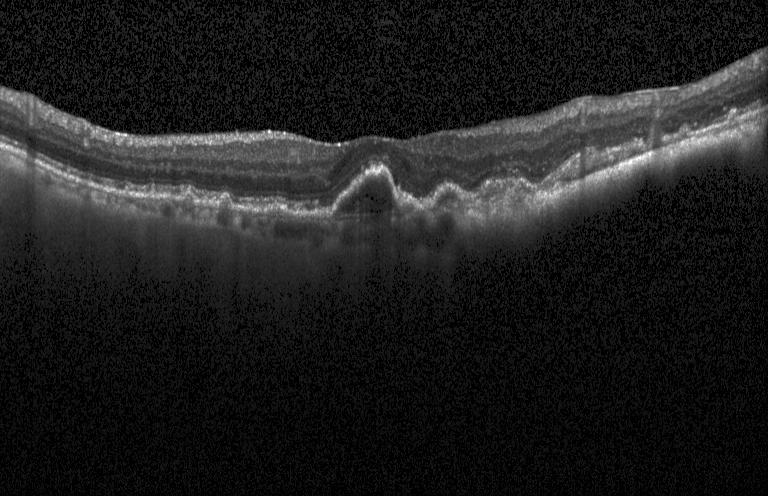
Spectral-domain OCT B-scan: choroidal neovascularization (CNV).